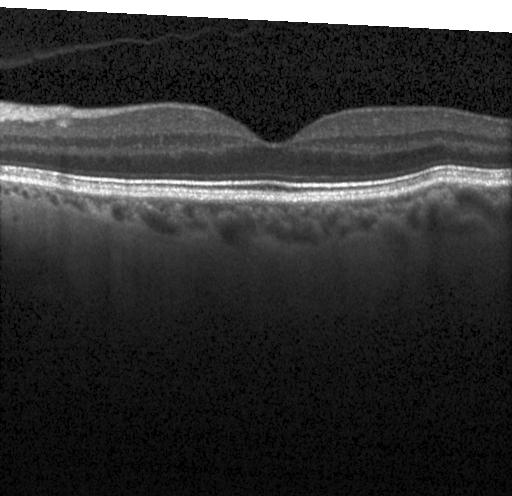
No choroidal neovascularization, no diabetic macular edema, and no drusen.